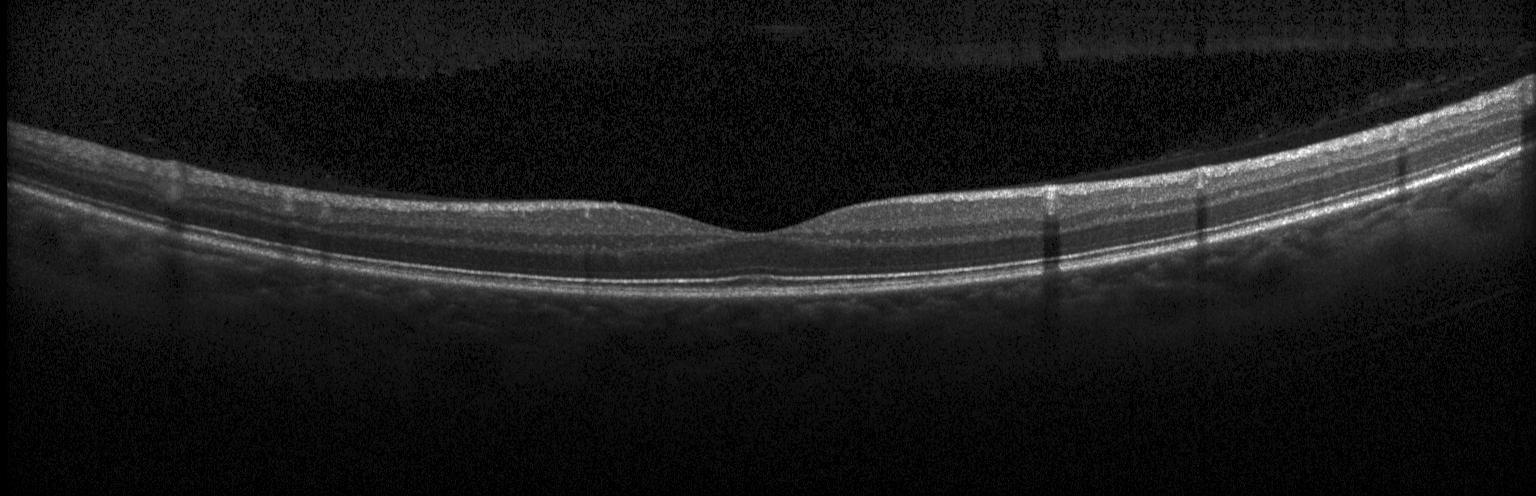 Spectral-domain optical coherence tomography. Acquired on a Heidelberg Spectralis. Horizontal scan through the fovea. Optical coherence tomography B-scan. Macular OCT: no evidence of choroidal neovascularization, diabetic macular edema, or drusen.